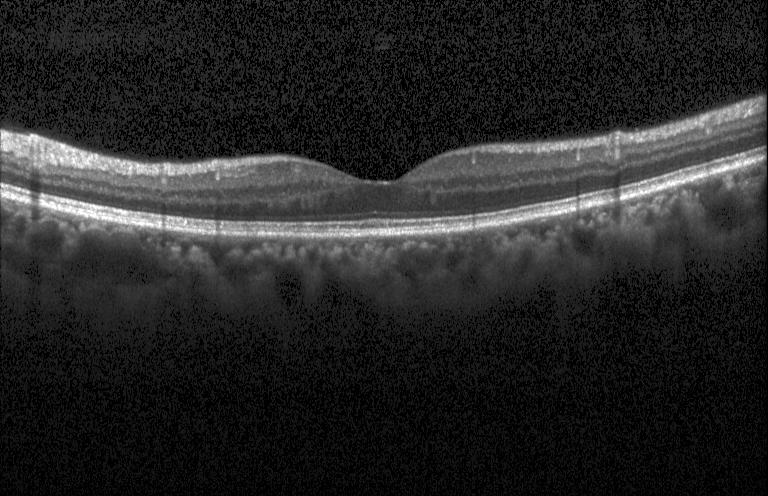 Fovea-centered; Heidelberg Spectralis OCT system; retinal OCT B-scan. Diagnosis: no choroidal neovascularization, no diabetic macular edema, and no drusen.